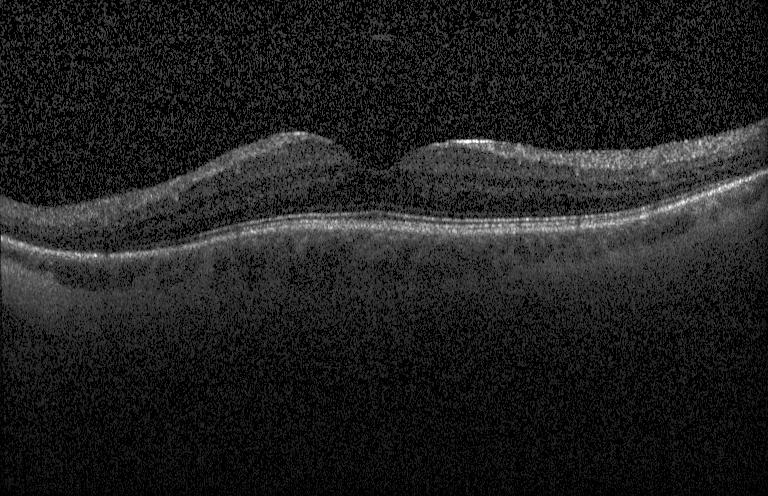 Retinal OCT cross-section · spectral-domain optical coherence tomography · horizontal scan through the fovea · instrument: Heidelberg Spectralis.
This B-scan demonstrates neither choroidal neovascularization, diabetic macular edema, nor drusen.